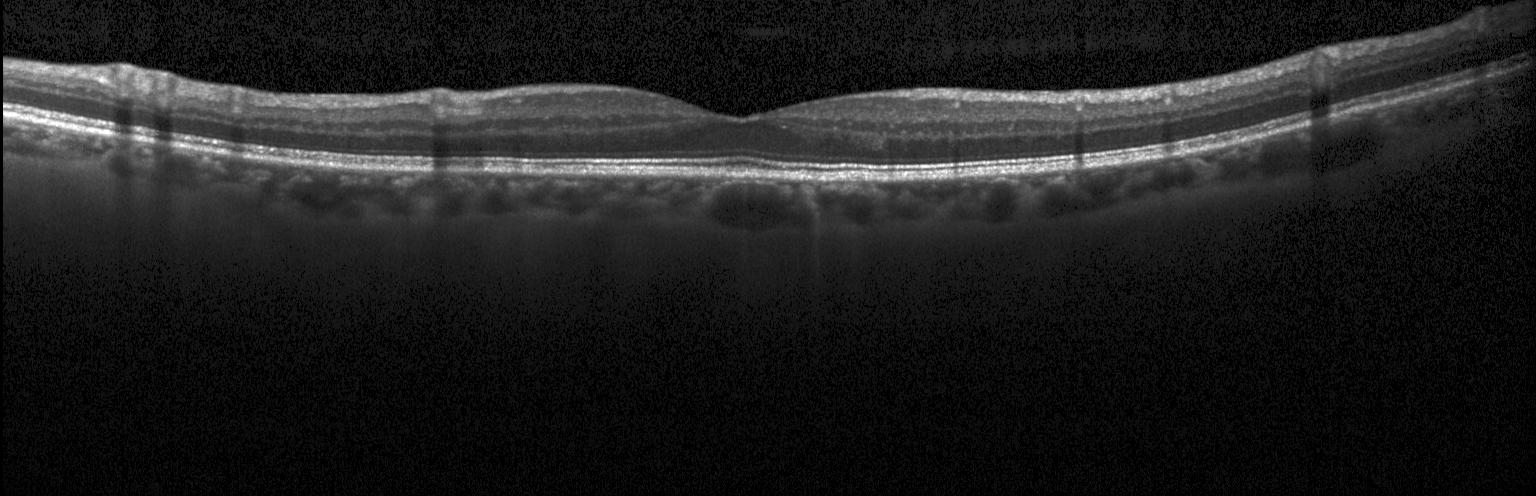 Macular scan. Optical coherence tomography scan. Spectral-domain OCT. This B-scan demonstrates no choroidal neovascularization, no diabetic macular edema, and no drusen.